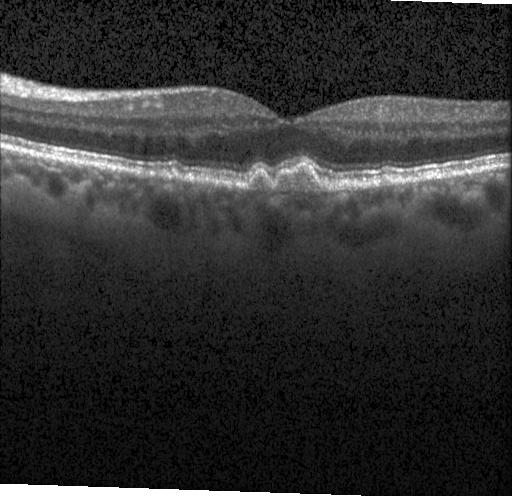

OCT line scan. Spectral-domain OCT. Diagnosis: multiple drusen.